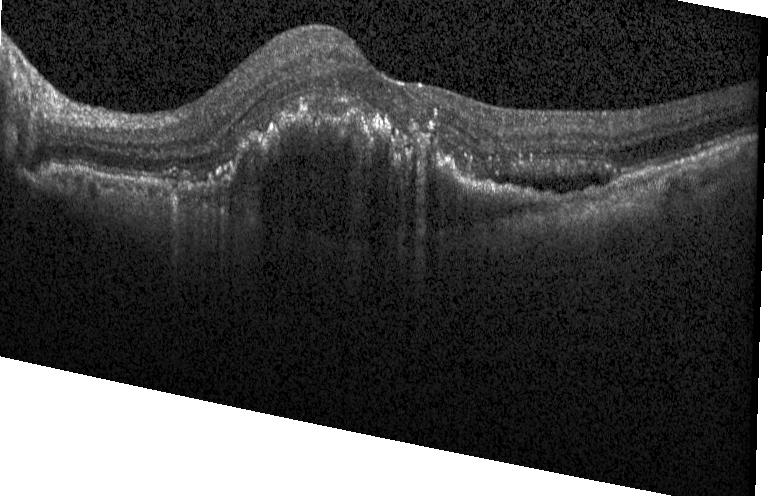
Fovea-centered · spectral-domain OCT · optical coherence tomography B-scan · Heidelberg Spectralis OCT system.
Finding: a choroidal neovascular membrane.